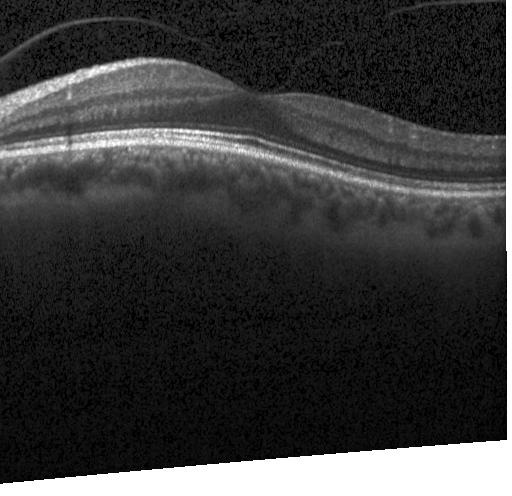
Impression: neither CNV, DME, nor drusen.